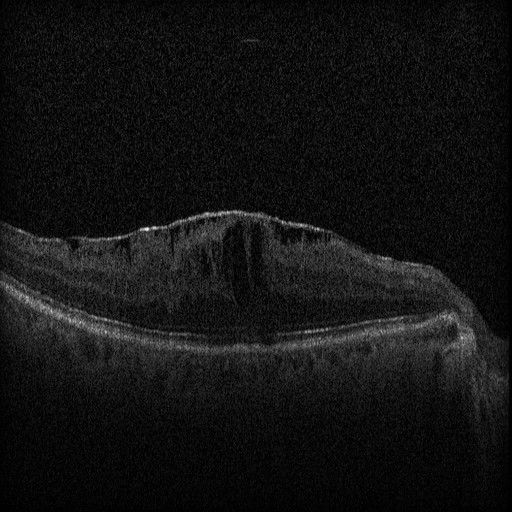

The scan shows diabetic macular edema.